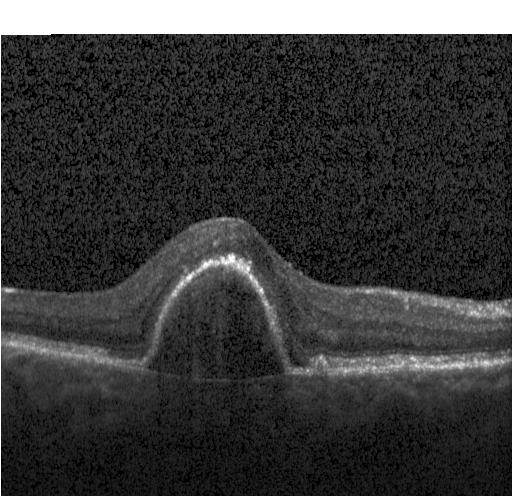 The scan shows CNV.